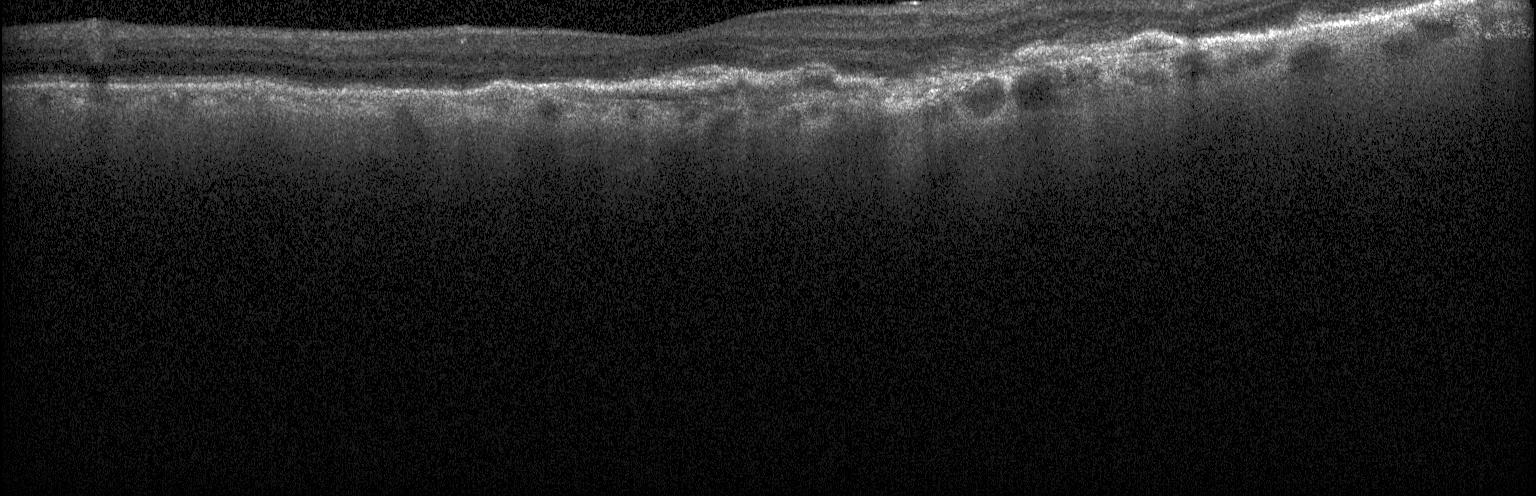 OCT B-scan · horizontal scan through the fovea
Diagnosis: choroidal neovascularization (CNV).